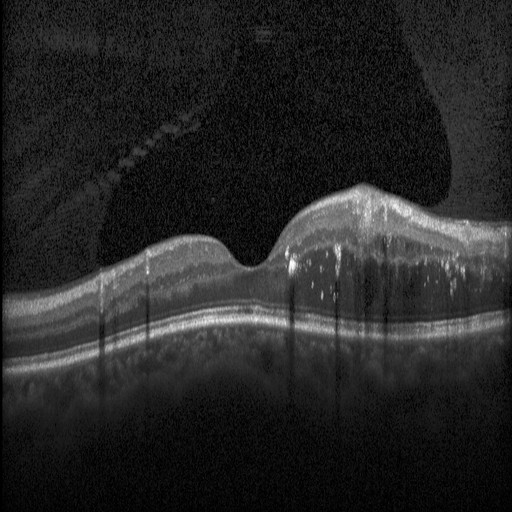

Optical coherence tomography B-scan.
Diagnosis: DME.